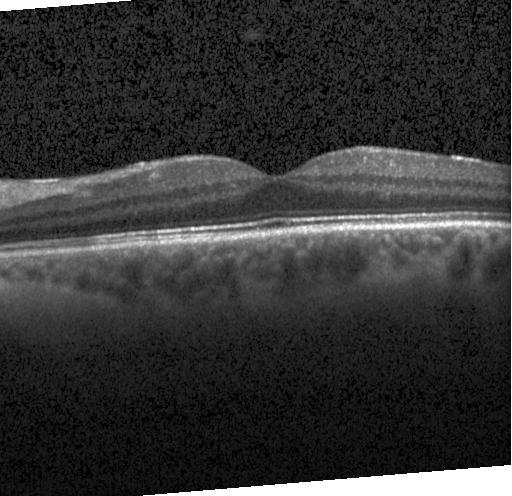
OCT B-scan. Acquired on a Heidelberg Spectralis. Fovea-centered. Spectral-domain optical coherence tomography.
Finding: neither CNV, DME, nor drusen.